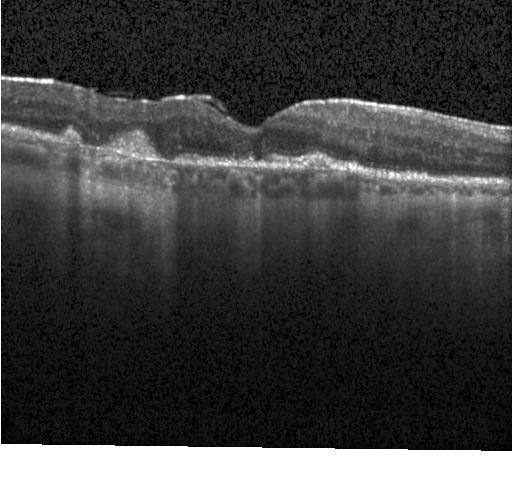
Retinal OCT B-scan. Spectral-domain OCT. Instrument: Heidelberg Spectralis
Assessment: a choroidal neovascular membrane.